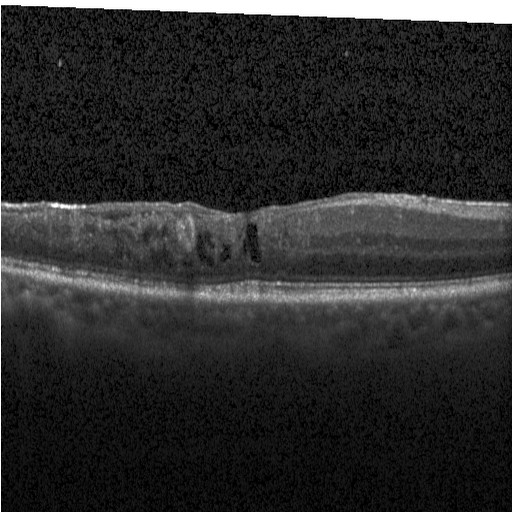
OCT B-scan showing diabetic macular edema.